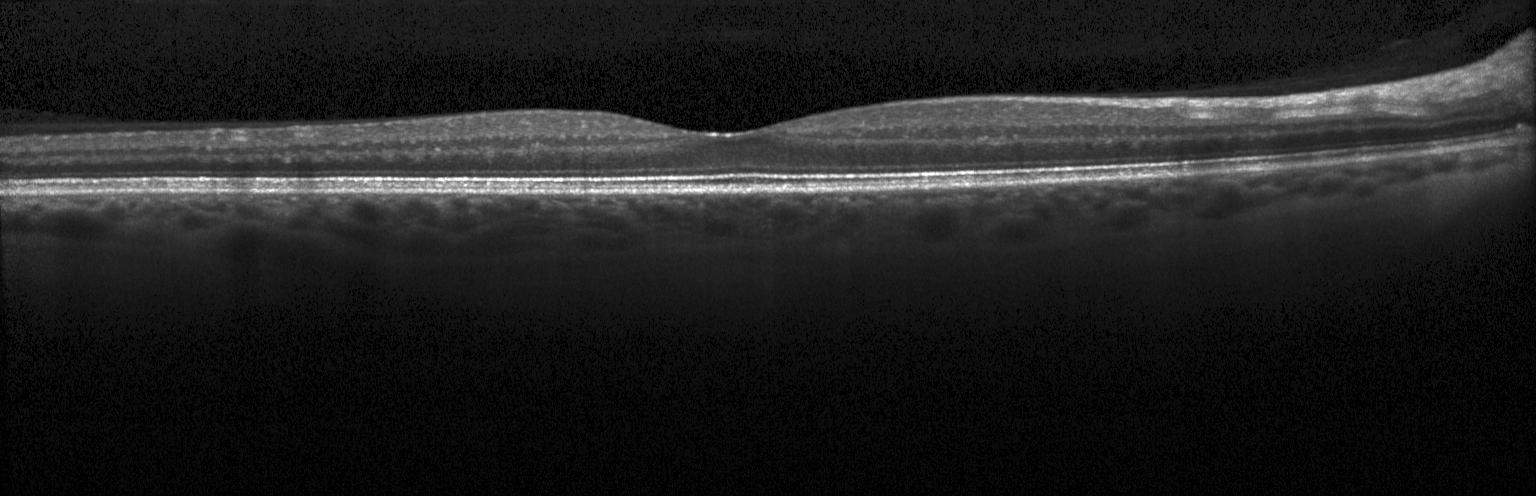

Acquired on a Heidelberg Spectralis. SD-OCT. Through the macula. OCT B-scan. No evidence of choroidal neovascularization, diabetic macular edema, or drusen.